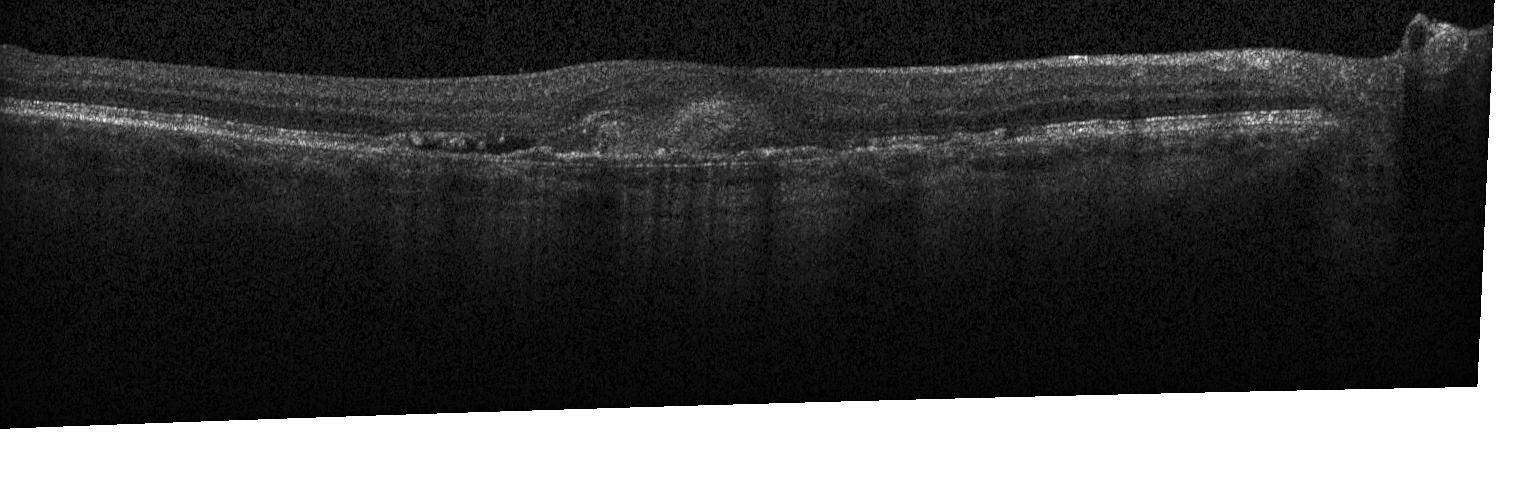
Instrument: Heidelberg Spectralis; OCT B-scan. Macular OCT: choroidal neovascularization (CNV).